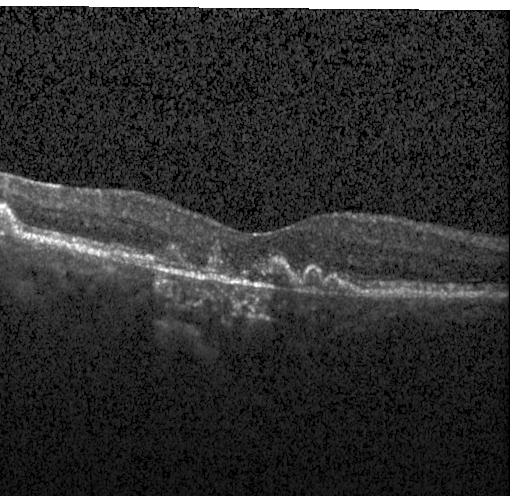

Optical coherence tomography scan
Assessment: a choroidal neovascular membrane.